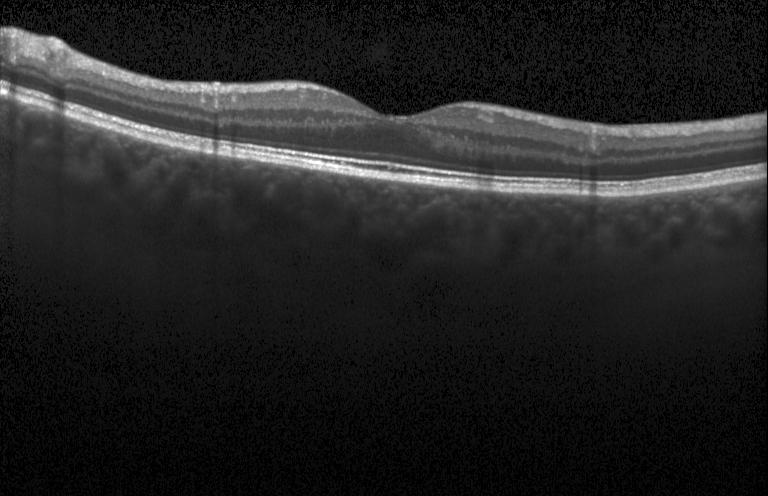

Centered on the fovea · OCT B-scan.
Dx: no choroidal neovascularization, diabetic macular edema, or drusen.